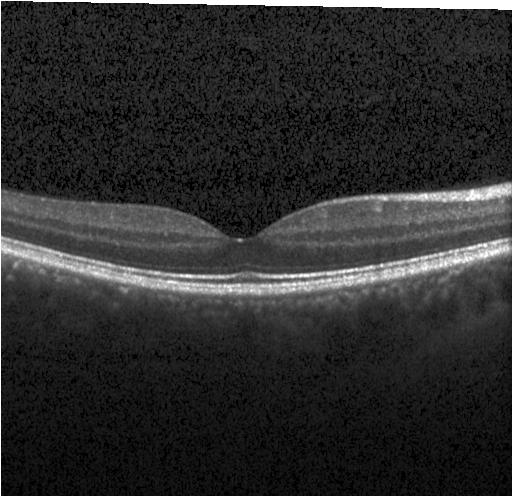
Neither CNV, DME, nor drusen.